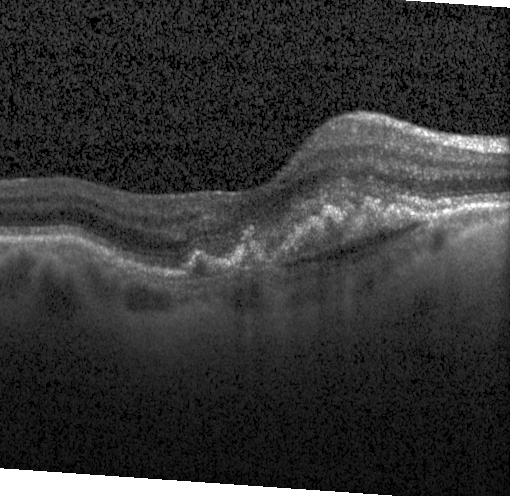

Finding: a choroidal neovascular membrane.